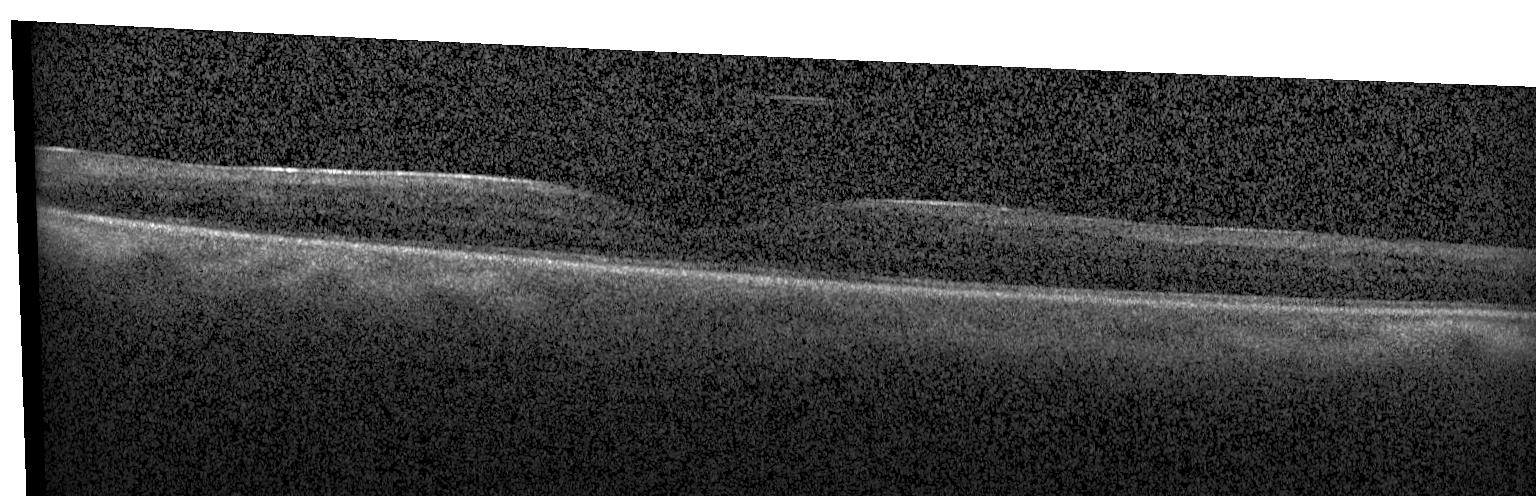

OCT line scan. Horizontal scan through the fovea. Instrument: Heidelberg Spectralis. Assessment: no CNV, DME, or drusen.